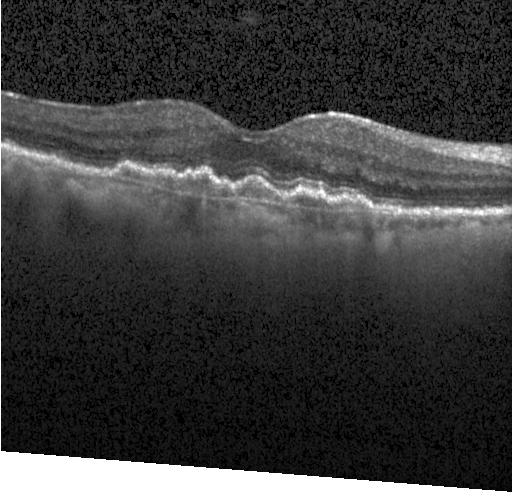

Retinal OCT B-scan.
This B-scan demonstrates choroidal neovascularization.